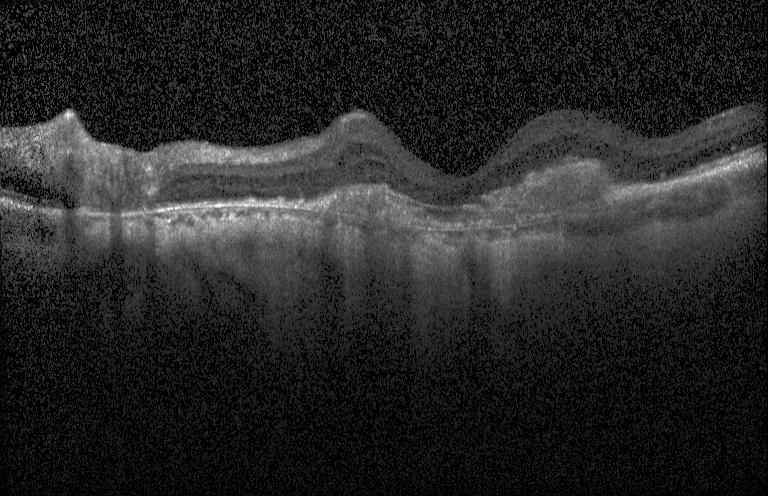 Horizontal scan through the fovea. Heidelberg Spectralis. Retinal OCT B-scan. Spectral-domain OCT.
Diagnosis: a choroidal neovascular membrane.